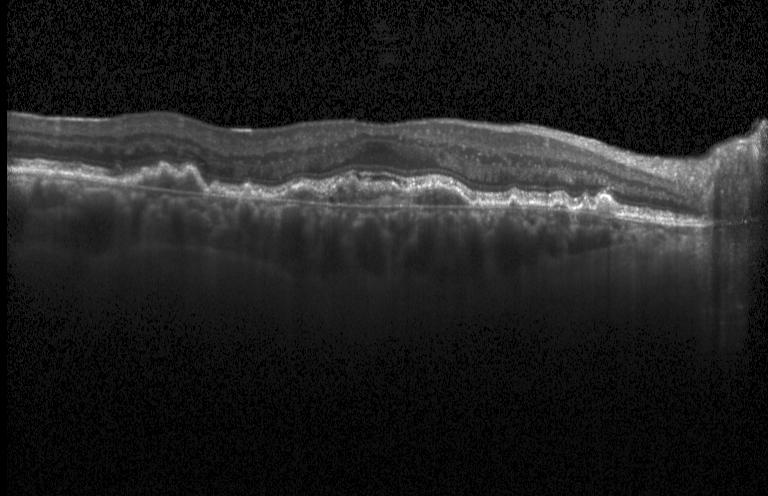

Spectral-domain OCT; retinal OCT B-scan; fovea-centered — Assessment: choroidal neovascularization.